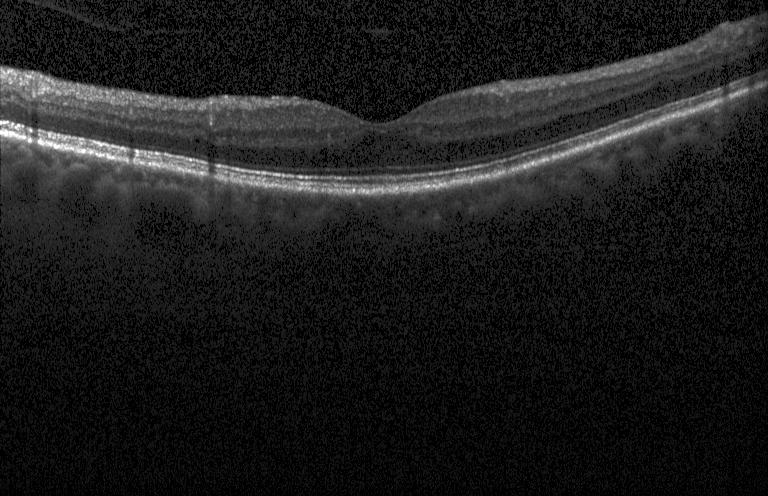

Dx: neither choroidal neovascularization, diabetic macular edema, nor drusen.